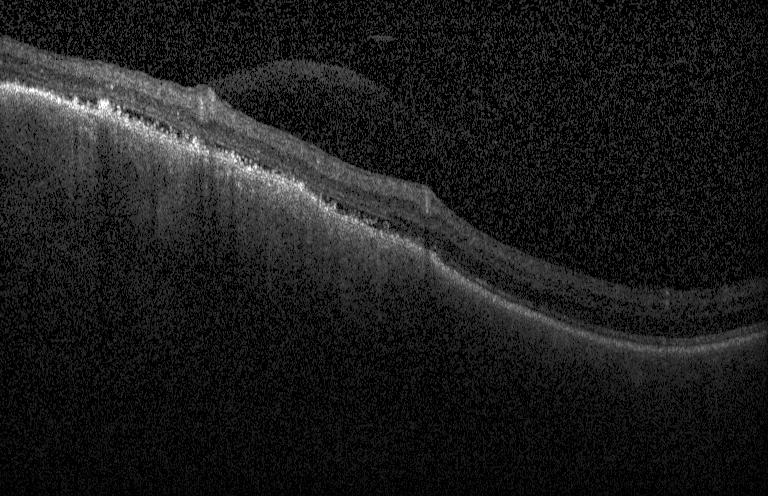
OCT B-scan · through the macula · SD-OCT
Assessment: a choroidal neovascular membrane.